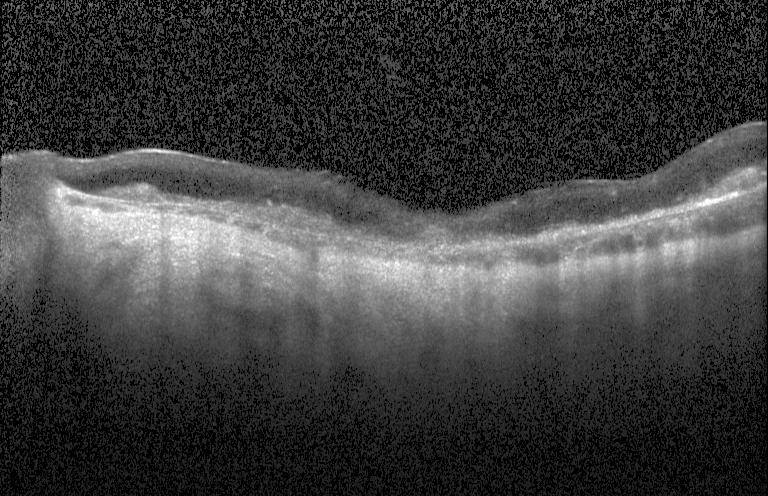
Impression: a choroidal neovascular membrane.